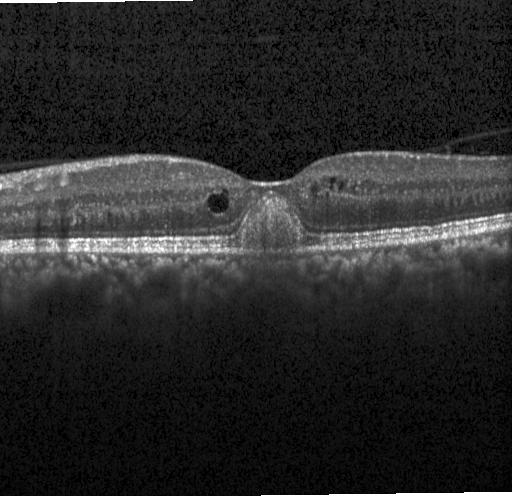 Finding: a choroidal neovascular membrane.